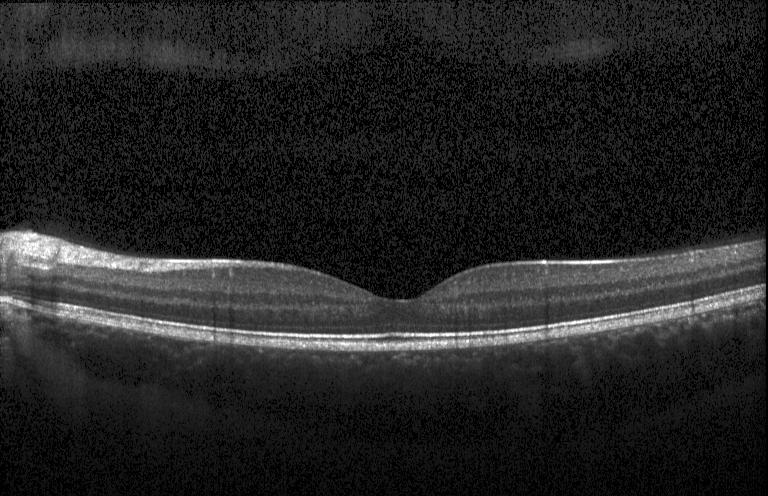 Optical coherence tomography B-scan, spectral-domain OCT, through the macula, instrument: Heidelberg Spectralis — The scan shows neither choroidal neovascularization, diabetic macular edema, nor drusen.